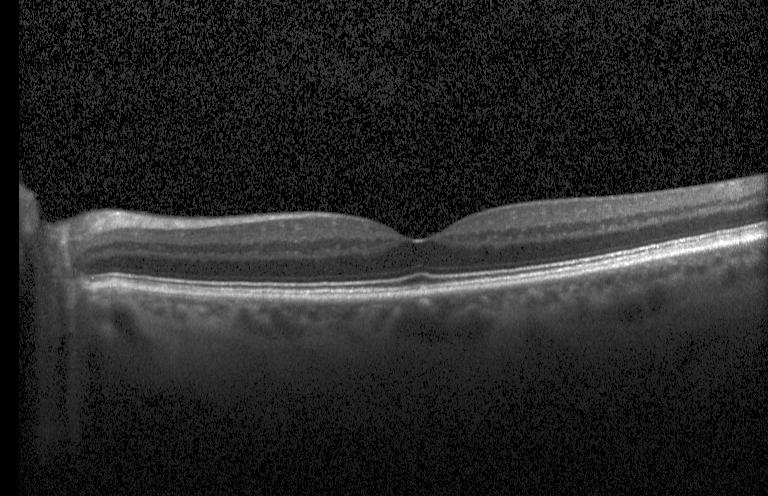
Spectral-domain optical coherence tomography. Centered on the fovea. OCT line scan.
Diagnosis: neither choroidal neovascularization, diabetic macular edema, nor drusen.